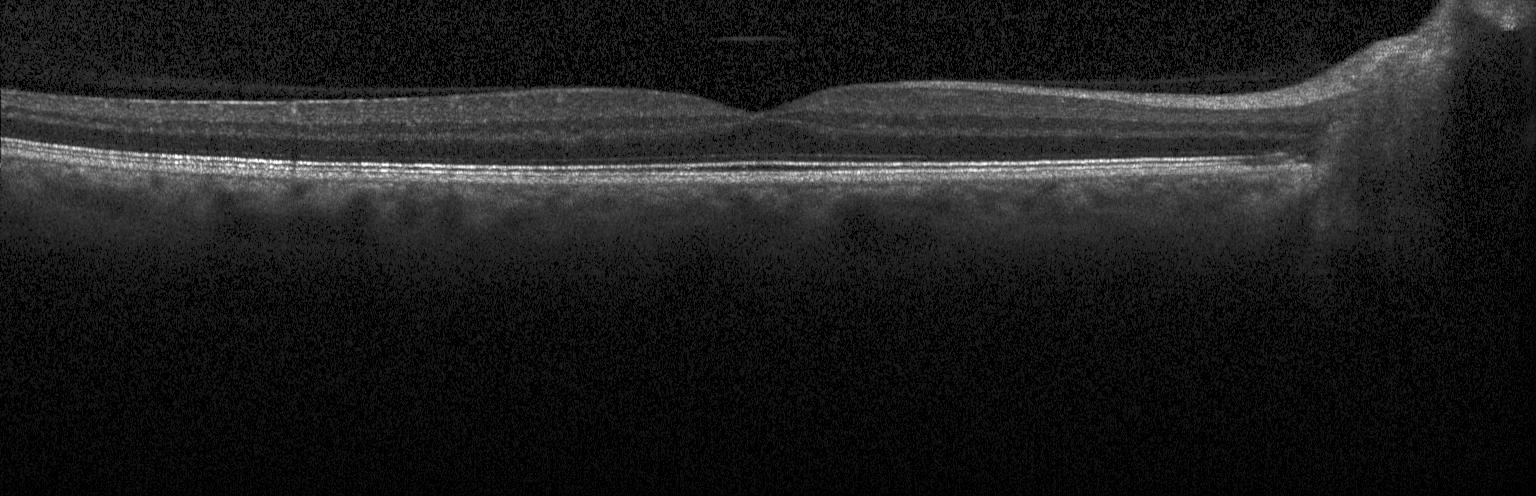
Finding: no evidence of CNV, DME, or drusen.